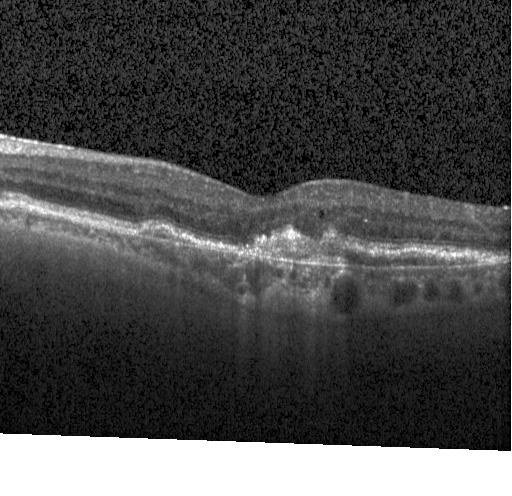
Spectral-domain OCT; acquired on a Heidelberg Spectralis; OCT B-scan.
A choroidal neovascular membrane.